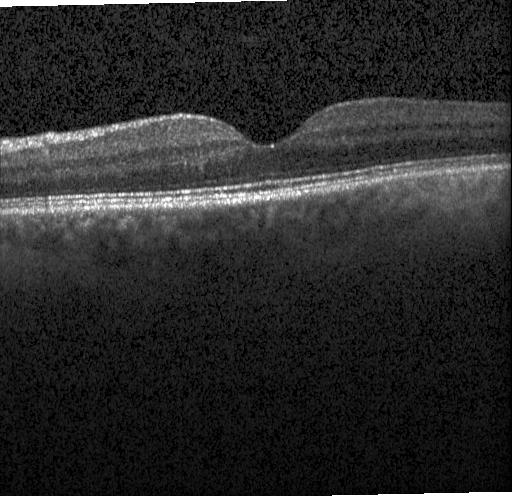
Acquired on a Heidelberg Spectralis, retinal OCT B-scan, fovea-centered, spectral-domain OCT. Impression: no choroidal neovascularization, no diabetic macular edema, and no drusen.